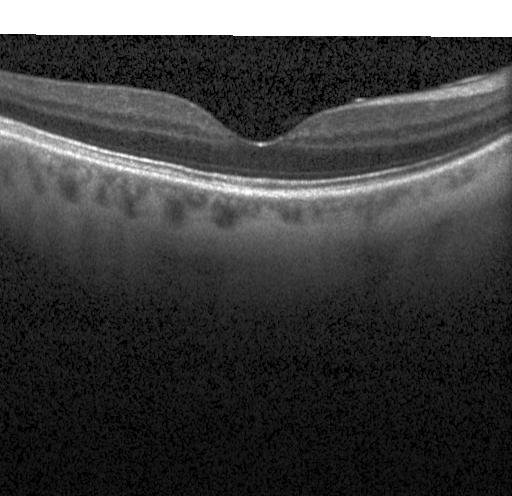

Retinal OCT cross-section — Dx: no CNV, no DME, and no drusen.